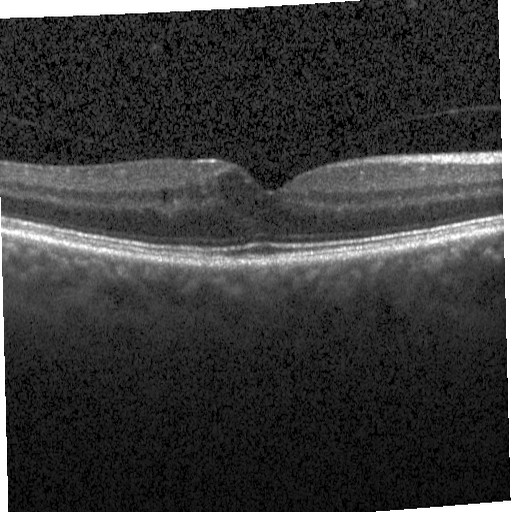
Optical coherence tomography B-scan · spectral-domain optical coherence tomography. Diagnosis: DME.